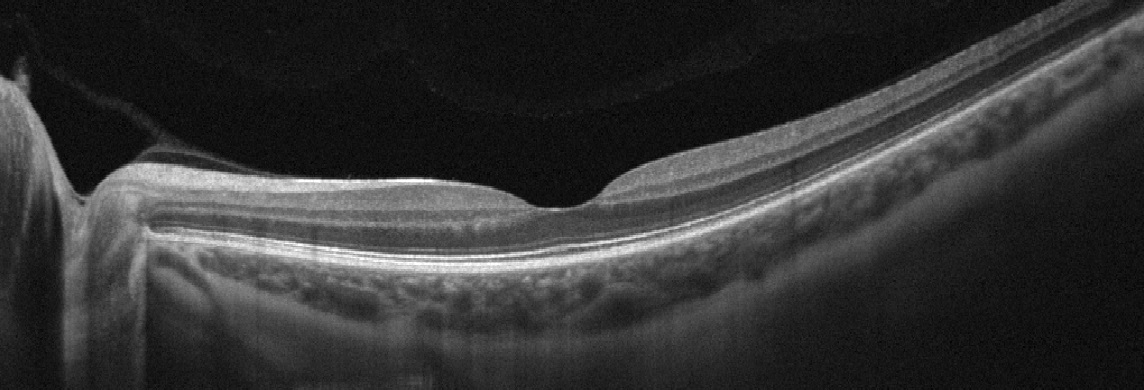
OCT B-scan, macular scan — Diagnosis: absence of AMD, DME, ERM, RAO, RVO, and vitreomacular interface disease.